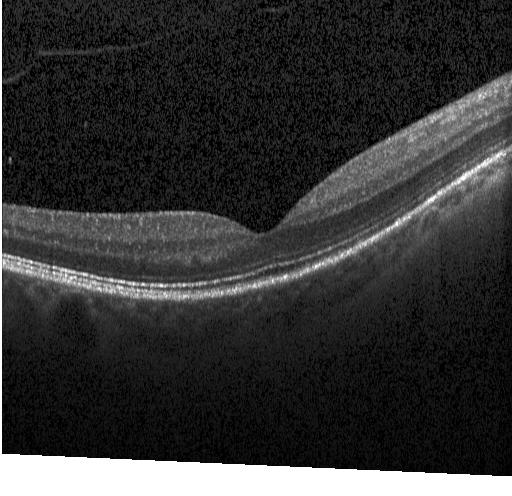 Centered on the fovea; spectral-domain optical coherence tomography; retinal OCT cross-section.
Dx: no choroidal neovascularization, no diabetic macular edema, and no drusen.